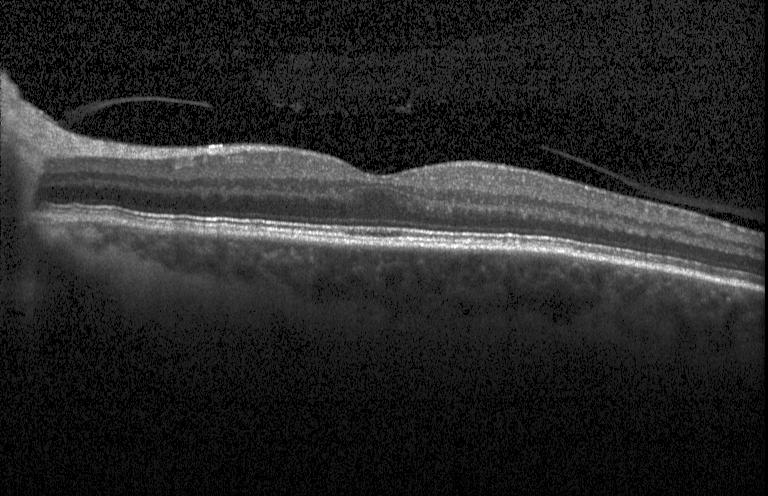

Assessment: no choroidal neovascularization, no diabetic macular edema, and no drusen.